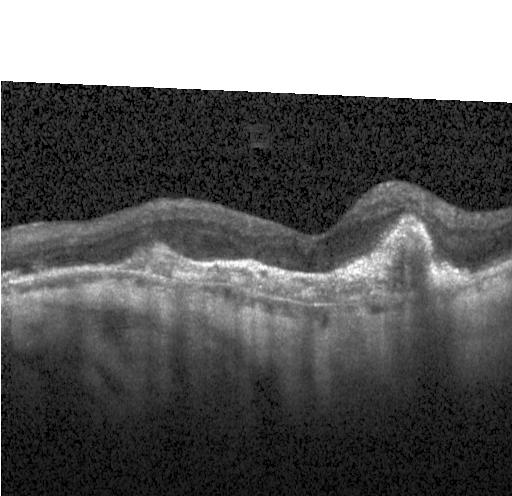

Heidelberg Spectralis OCT system · OCT line scan · through the macula — Finding: choroidal neovascularization.